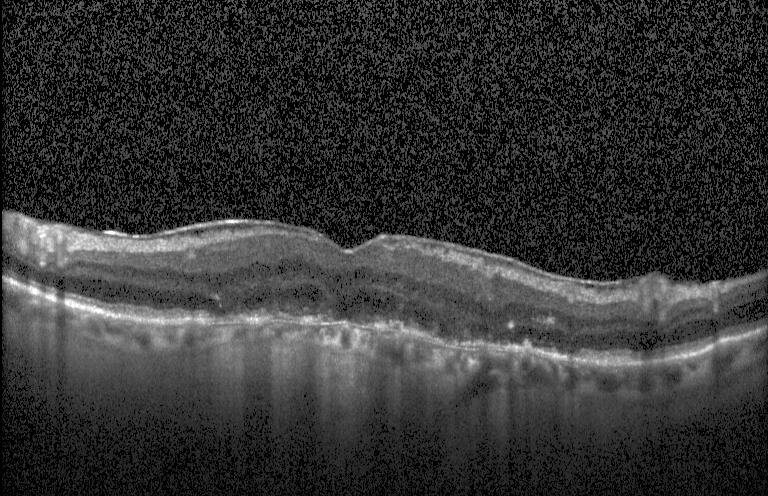
Heidelberg Spectralis, macular scan, retinal OCT cross-section, spectral-domain OCT. The scan shows CNV.